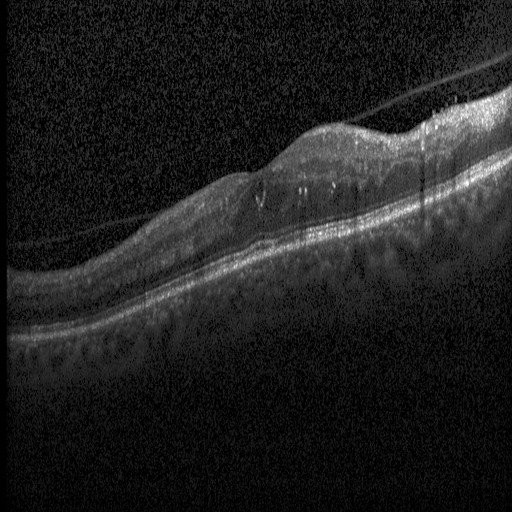
This B-scan demonstrates diabetic macular edema (DME).